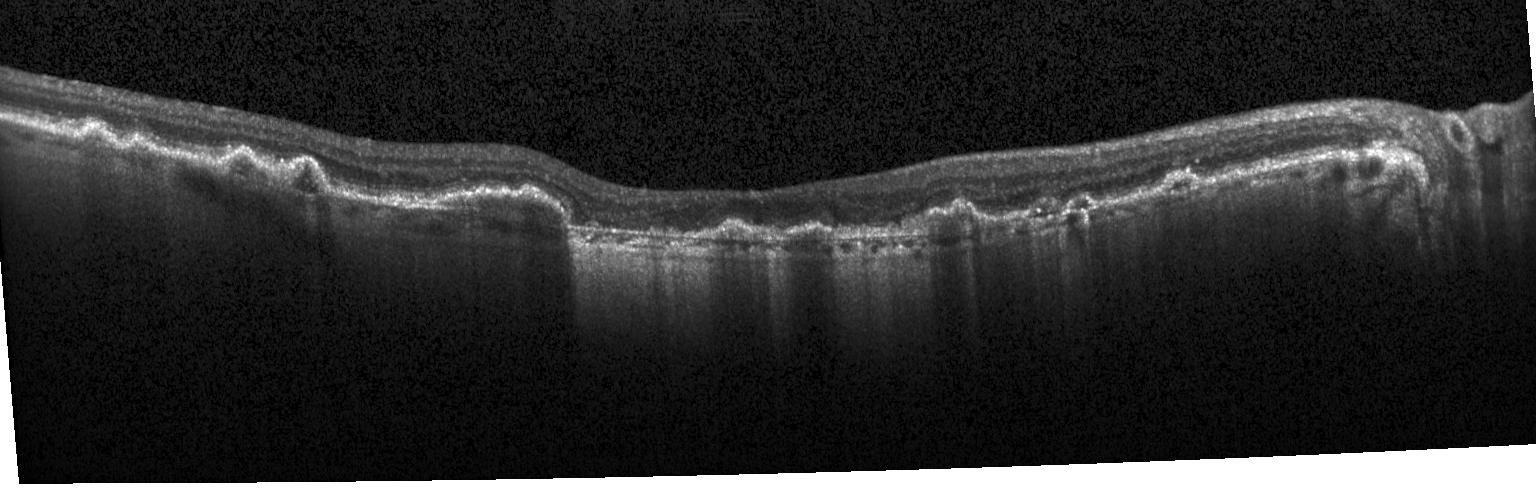

Optical coherence tomography B-scan · through the macula · Heidelberg Spectralis OCT system. Dx: a choroidal neovascular membrane.